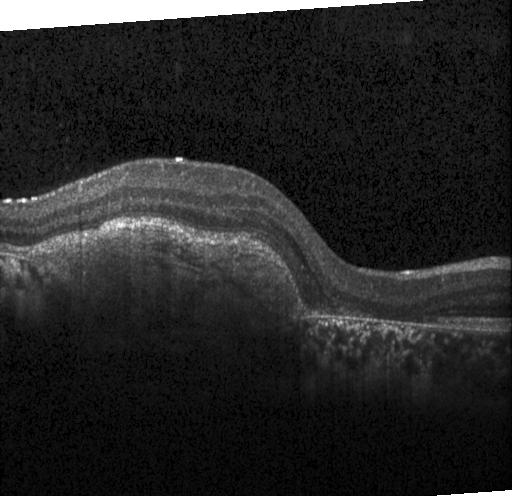
Centered on the fovea; OCT B-scan; spectral-domain optical coherence tomography; Heidelberg Spectralis. Assessment: a choroidal neovascular membrane.